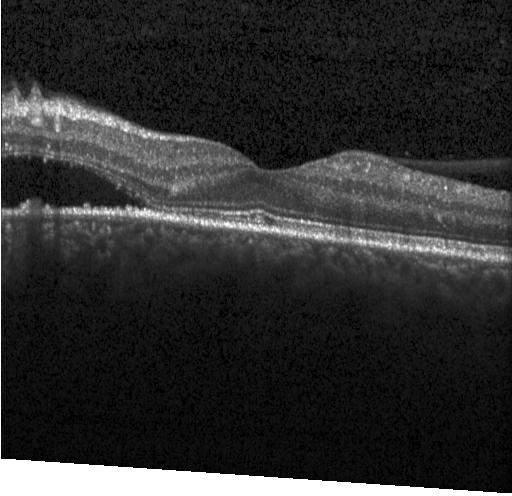
Optical coherence tomography scan — Impression: a choroidal neovascular membrane.